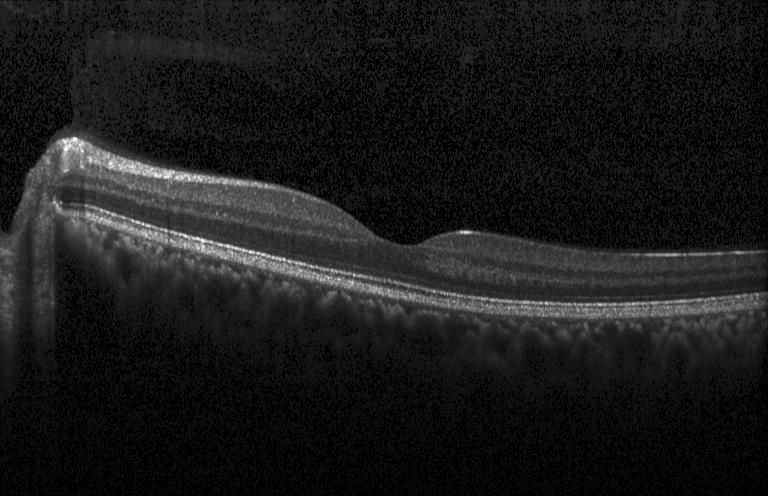

Assessment: no choroidal neovascularization, diabetic macular edema, or drusen.